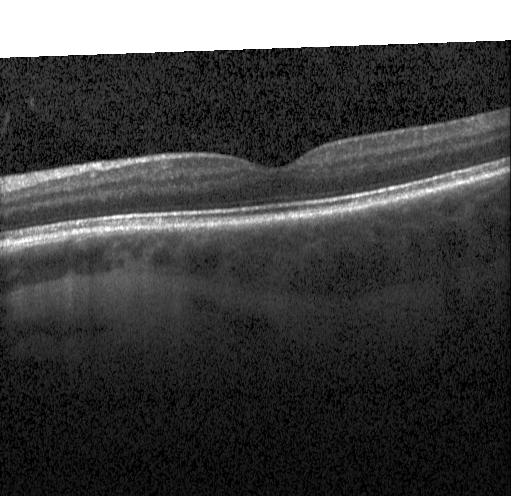 Spectral-domain optical coherence tomography · retinal OCT cross-section. Impression: no choroidal neovascularization, diabetic macular edema, or drusen.